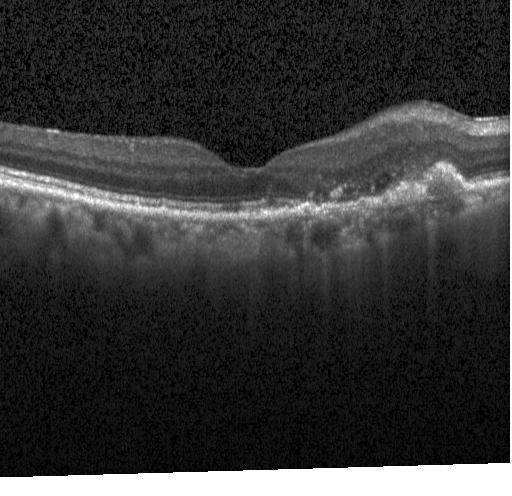

Optical coherence tomography B-scan.
Diagnosis: a choroidal neovascular membrane.